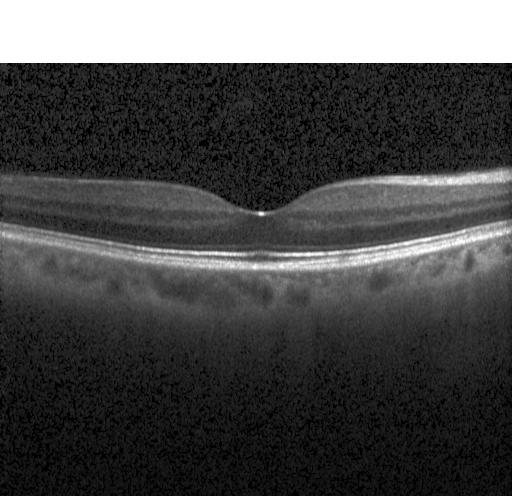
Spectral-domain OCT. Acquired on a Heidelberg Spectralis. OCT B-scan. Macular scan — Impression: neither CNV, DME, nor drusen.